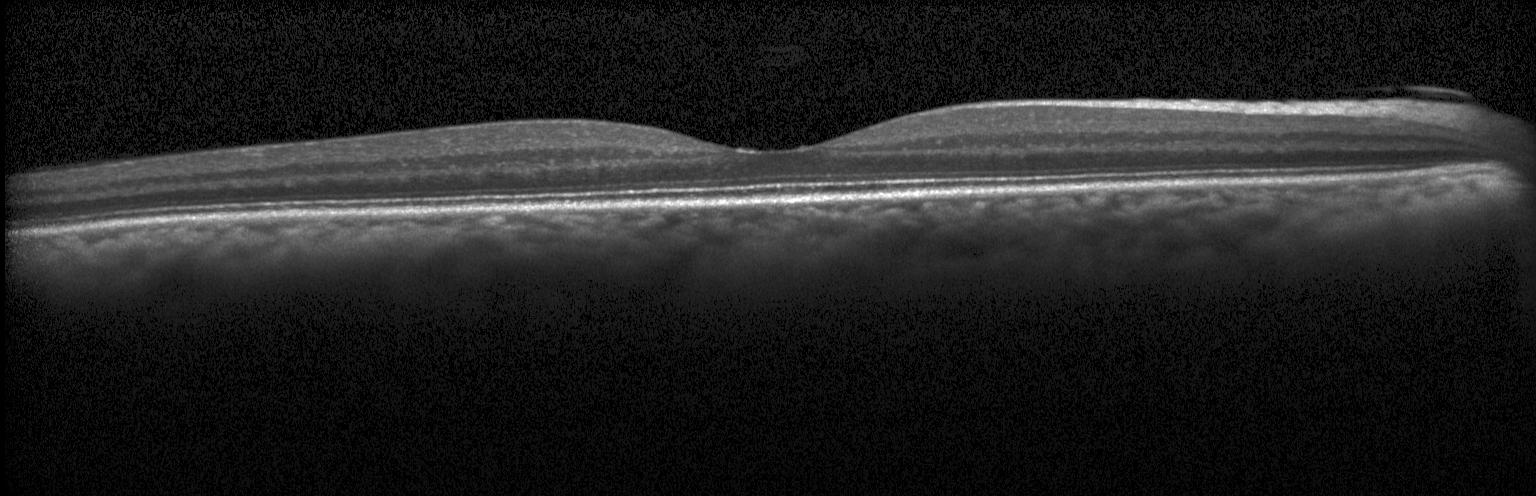
Macular scan, optical coherence tomography scan, instrument: Heidelberg Spectralis.
OCT finding: no evidence of CNV, DME, or drusen.